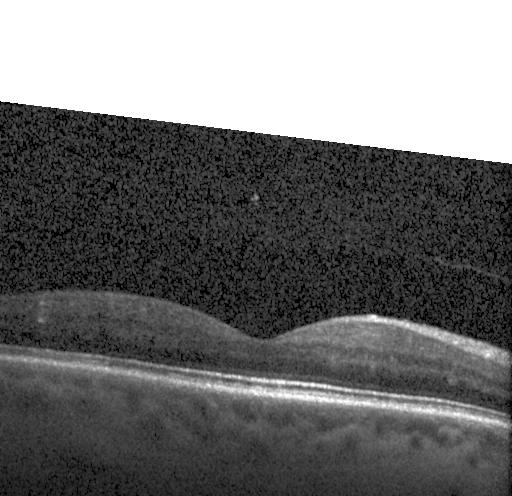
Optical coherence tomography scan — No choroidal neovascularization, diabetic macular edema, or drusen.